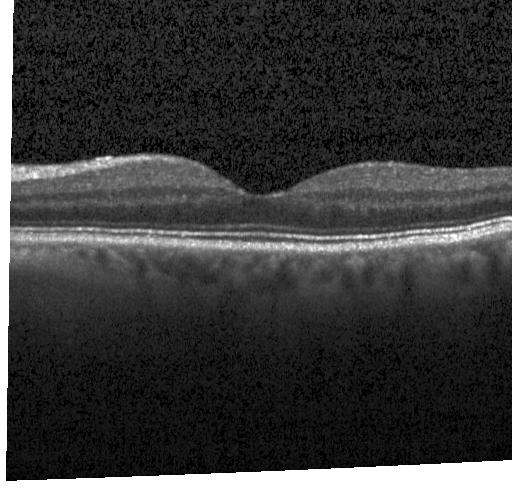
Dx: no evidence of choroidal neovascularization, diabetic macular edema, or drusen.